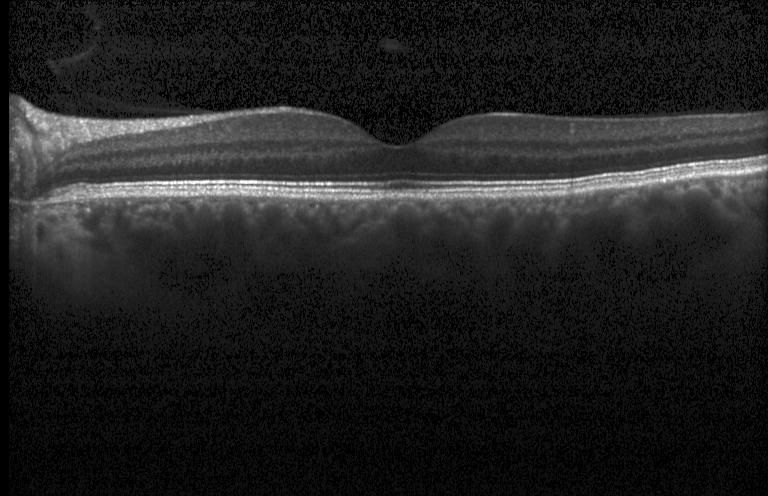

SD-OCT · optical coherence tomography scan · acquired on a Heidelberg Spectralis · fovea-centered. OCT finding: neither choroidal neovascularization, diabetic macular edema, nor drusen.